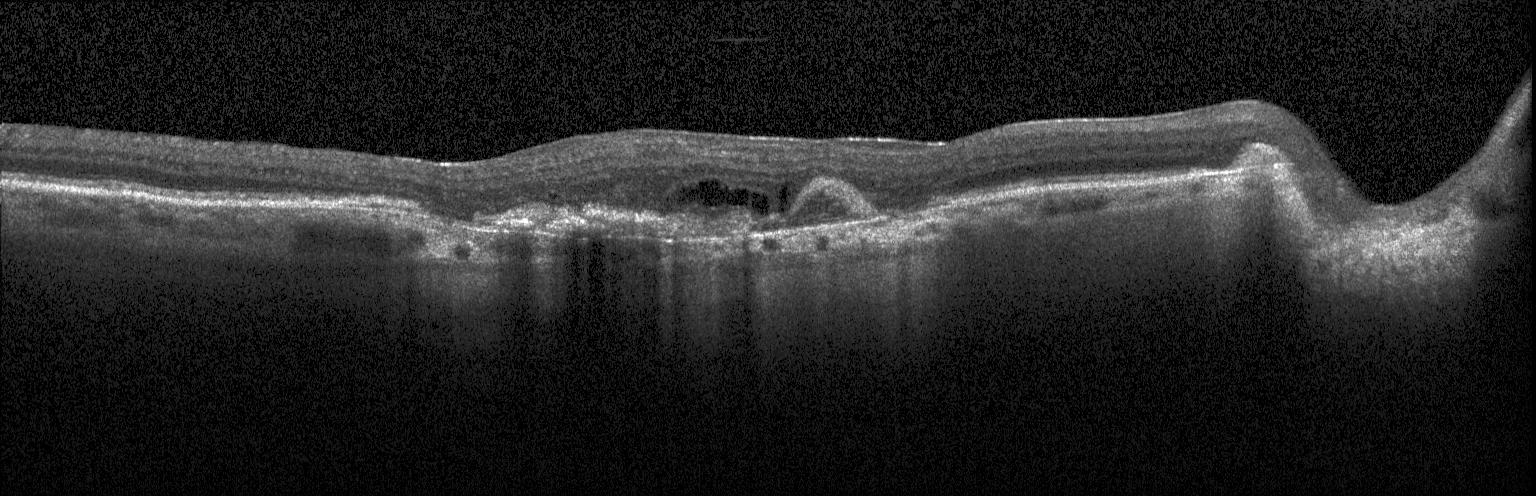

Through the macula · SD-OCT · Heidelberg Spectralis · retinal OCT B-scan.
This B-scan demonstrates choroidal neovascularization (CNV).